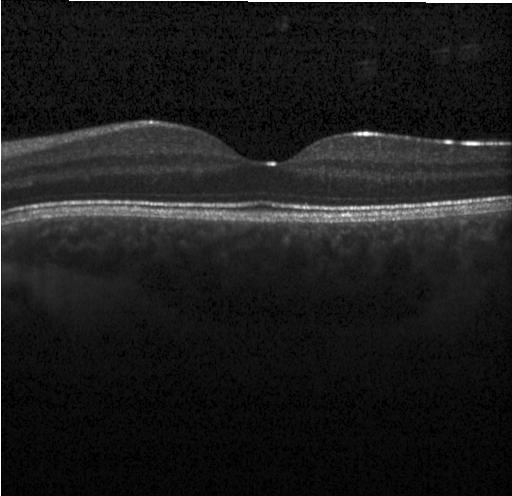 Horizontal scan through the fovea; Heidelberg Spectralis OCT system; optical coherence tomography scan; spectral-domain optical coherence tomography — The scan shows neither choroidal neovascularization, diabetic macular edema, nor drusen.